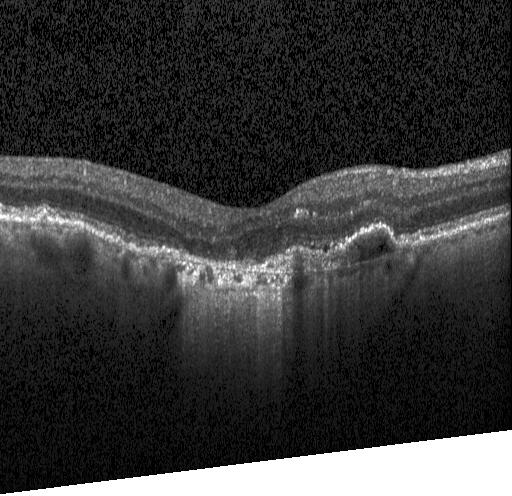 Retinal OCT B-scan.
The scan shows a choroidal neovascular membrane.